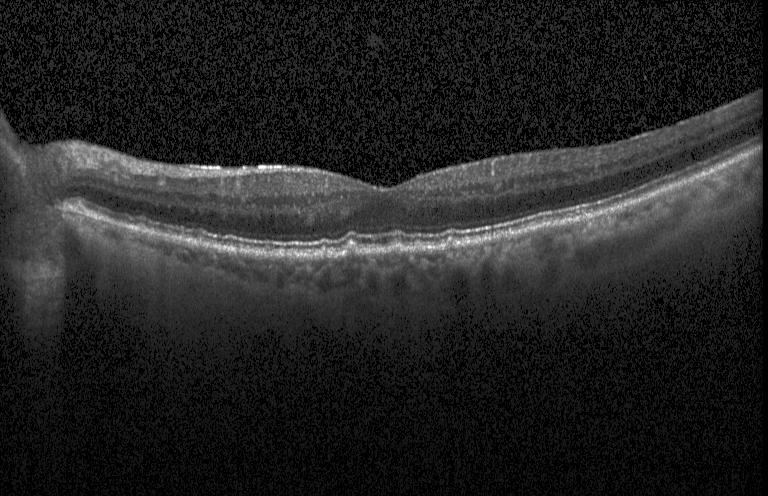 OCT B-scan · acquired on a Heidelberg Spectralis — Assessment: drusen.